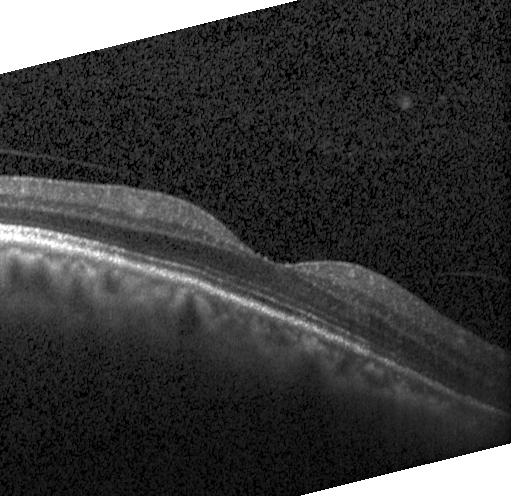
OCT line scan
Diagnosis: no CNV, DME, or drusen.